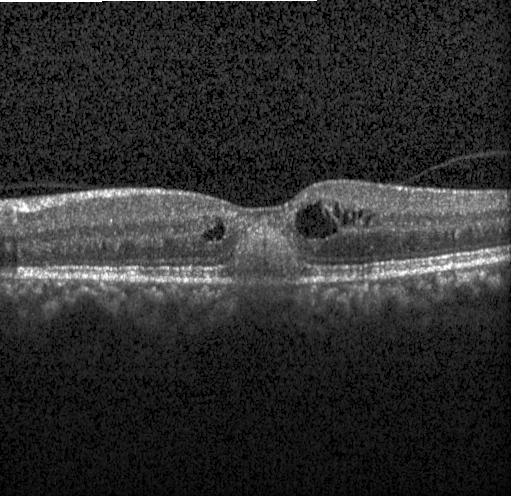
Macular OCT: a choroidal neovascular membrane.